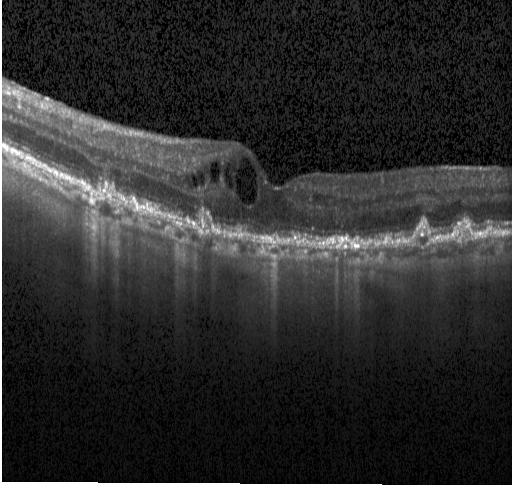

Diagnosis: a choroidal neovascular membrane.